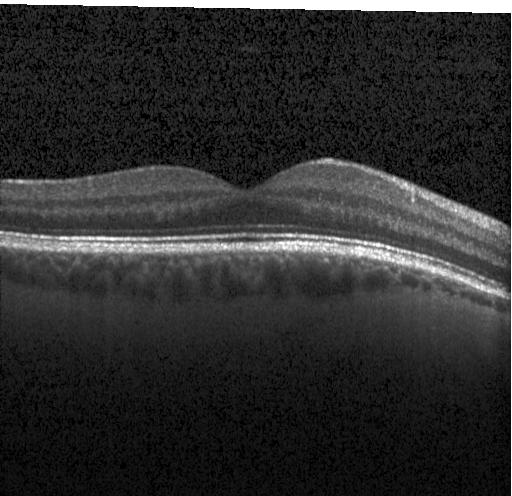

Optical coherence tomography scan, Heidelberg Spectralis OCT system, fovea-centered — Assessment: no choroidal neovascularization, diabetic macular edema, or drusen.